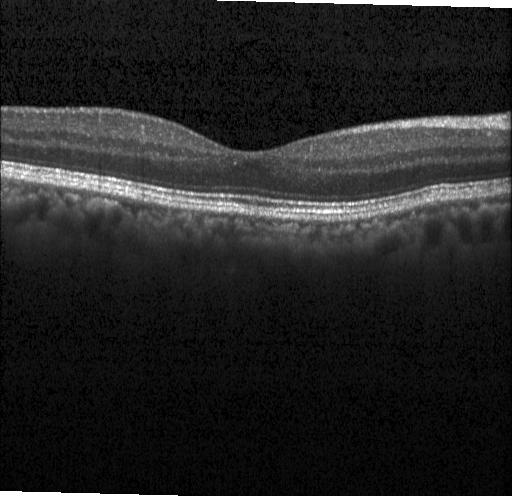
The scan shows no CNV, no DME, and no drusen.